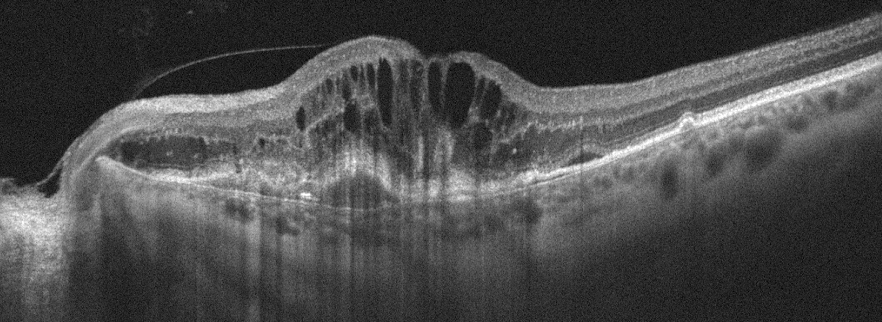

OCT B-scan showing age-related macular degeneration (AMD).